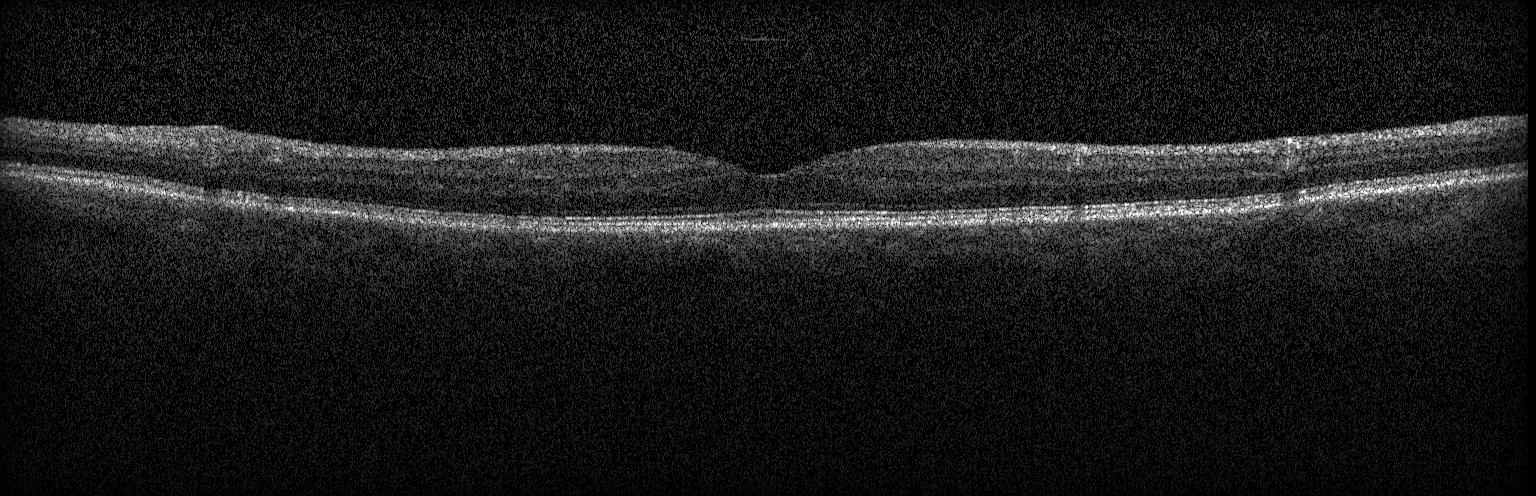 Spectral-domain OCT, OCT B-scan, macular scan.
No evidence of CNV, DME, or drusen.